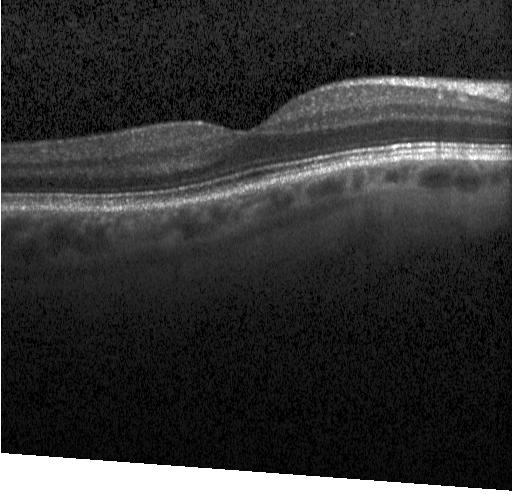
Assessment: no choroidal neovascularization, no diabetic macular edema, and no drusen.